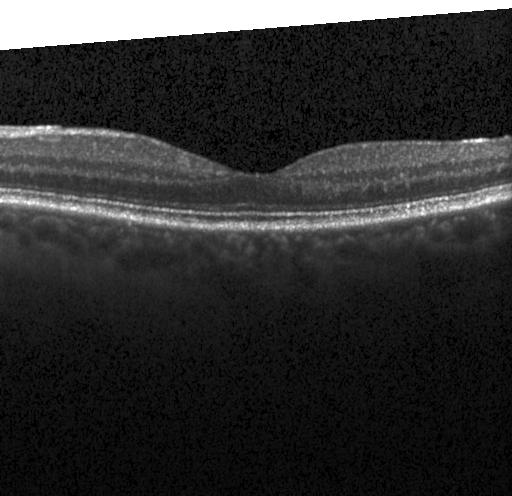
OCT finding: no choroidal neovascularization, no diabetic macular edema, and no drusen.